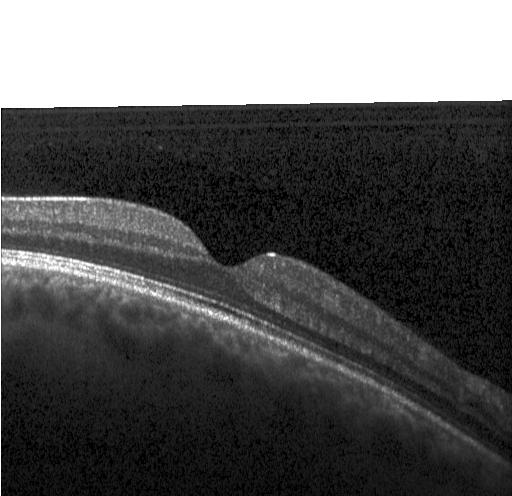

Macular scan, optical coherence tomography B-scan, Heidelberg Spectralis OCT system
Impression: no choroidal neovascularization, no diabetic macular edema, and no drusen.